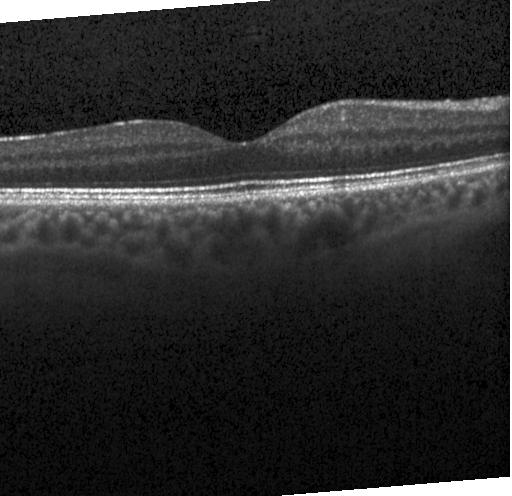
Retinal OCT B-scan — Finding: neither choroidal neovascularization, diabetic macular edema, nor drusen.